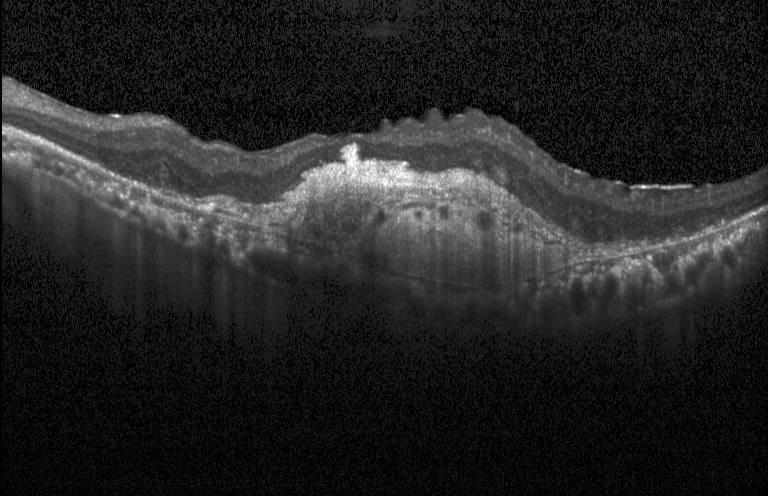
Dx: a choroidal neovascular membrane.